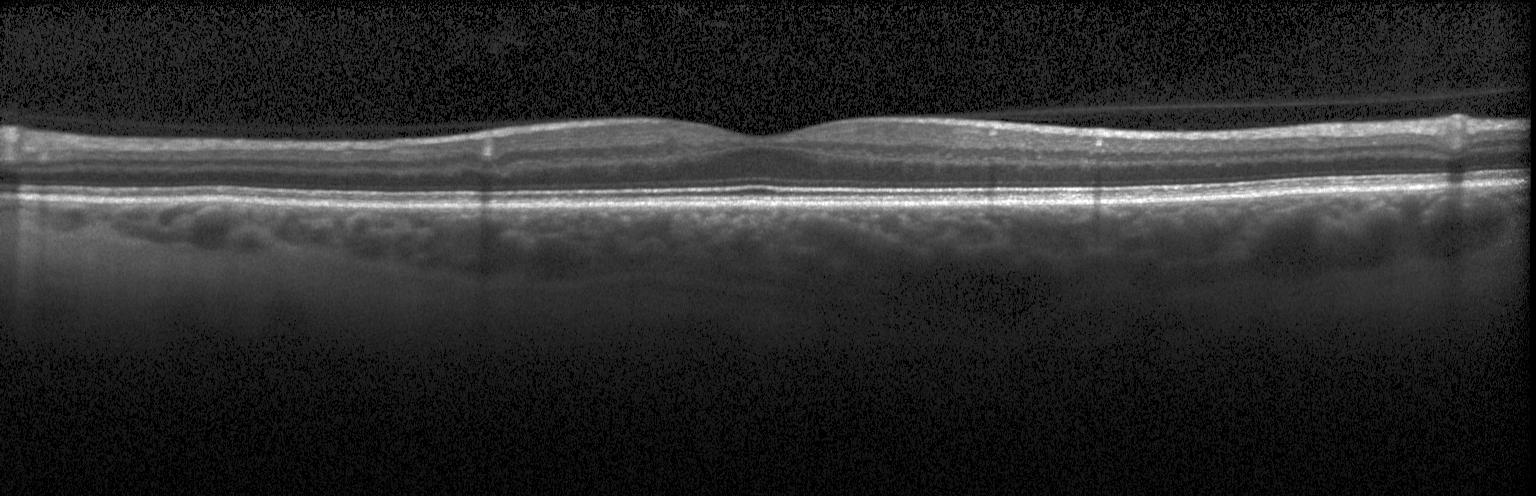
OCT B-scan; fovea-centered. Impression: no choroidal neovascularization, diabetic macular edema, or drusen.